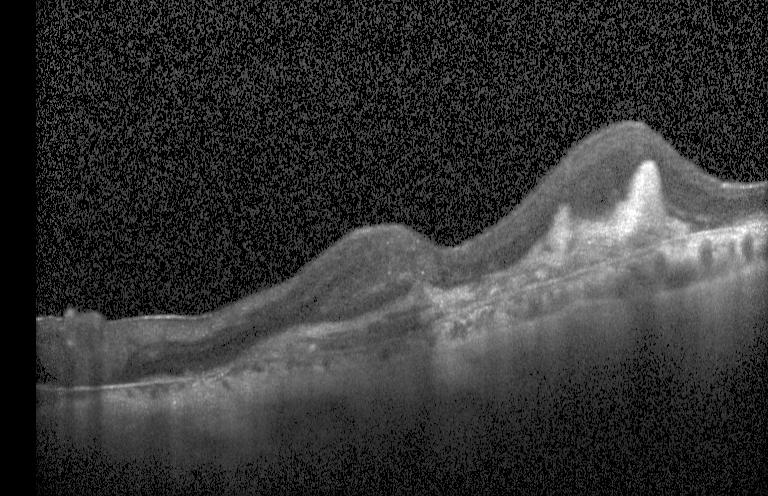
OCT line scan, acquired on a Heidelberg Spectralis — Choroidal neovascularization.